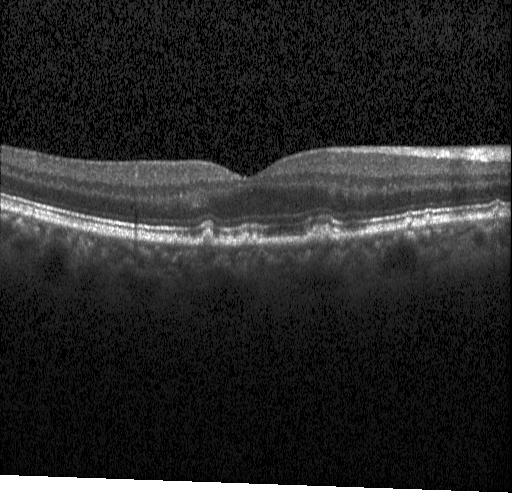
Impression: drusen.